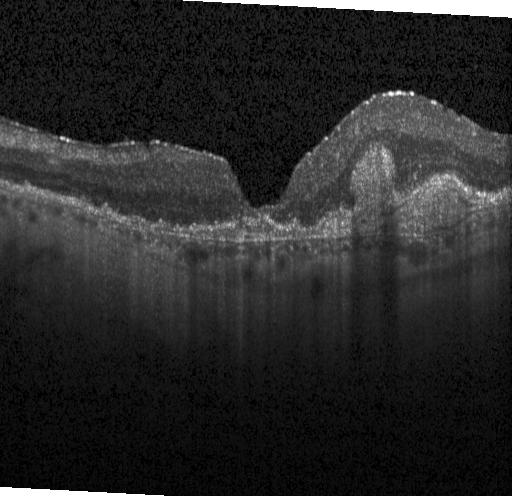

Optical coherence tomography scan, spectral-domain OCT, macular scan, acquired on a Heidelberg Spectralis. Finding: a choroidal neovascular membrane.